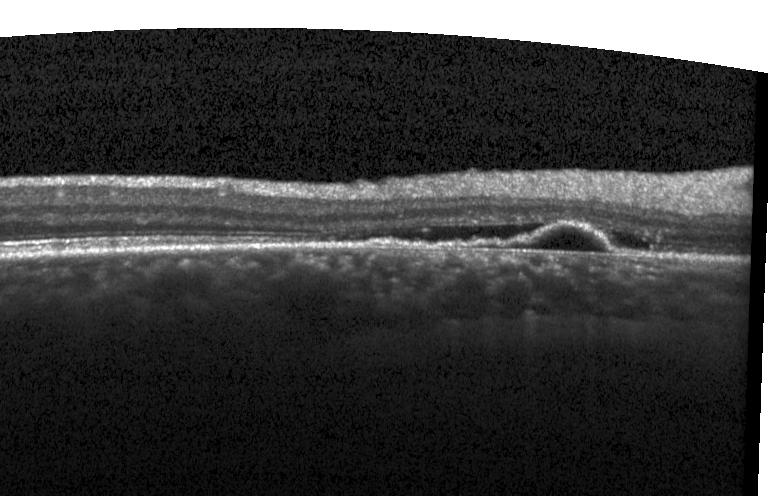 OCT line scan, centered on the fovea, acquired on a Heidelberg Spectralis.
Finding: CNV.